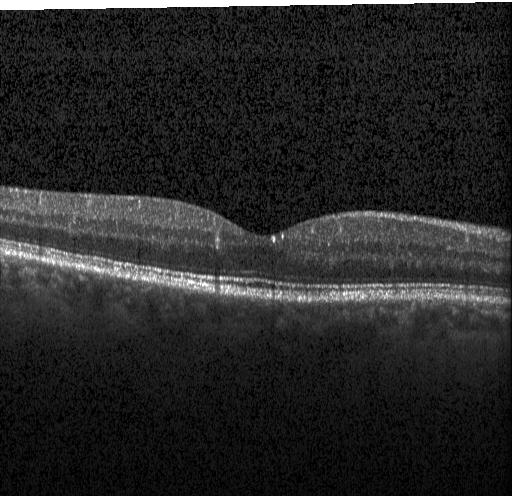
Macular OCT: no choroidal neovascularization, no diabetic macular edema, and no drusen.